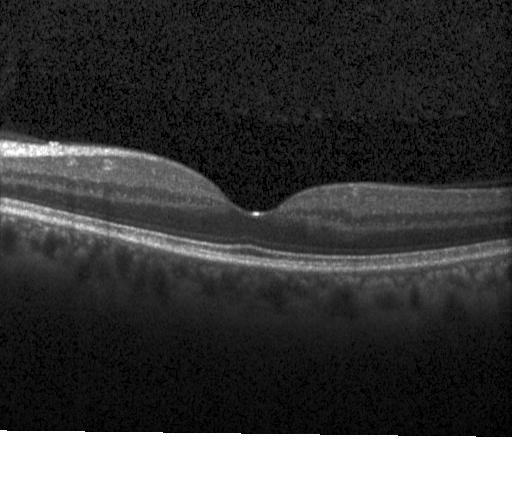

Diagnosis: no choroidal neovascularization, no diabetic macular edema, and no drusen.